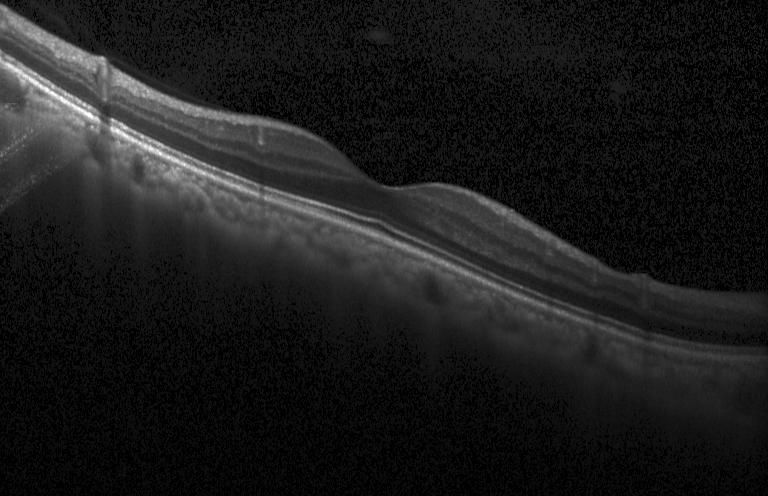 Optical coherence tomography scan; fovea-centered; acquired on a Heidelberg Spectralis
The scan shows no choroidal neovascularization, no diabetic macular edema, and no drusen.